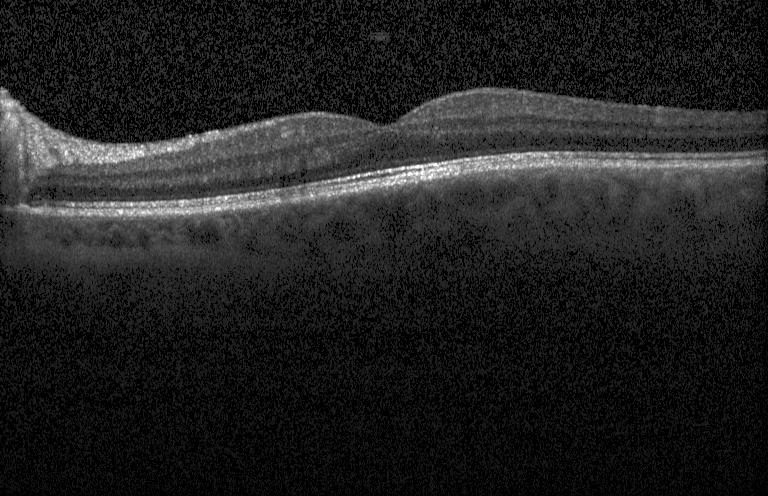
Macular OCT demonstrating no choroidal neovascularization, no diabetic macular edema, and no drusen.